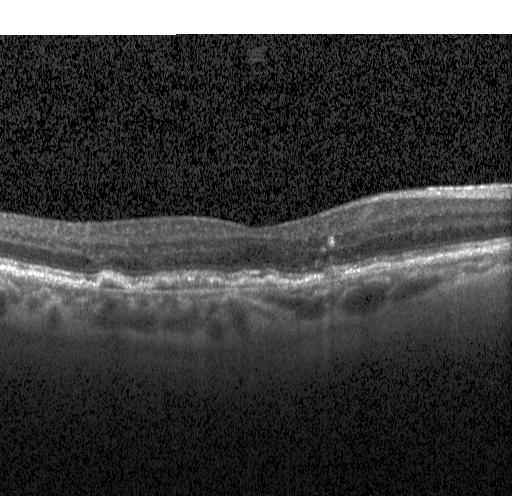 Optical coherence tomography scan; acquired on a Heidelberg Spectralis; SD-OCT; centered on the fovea. Macular OCT: CNV.